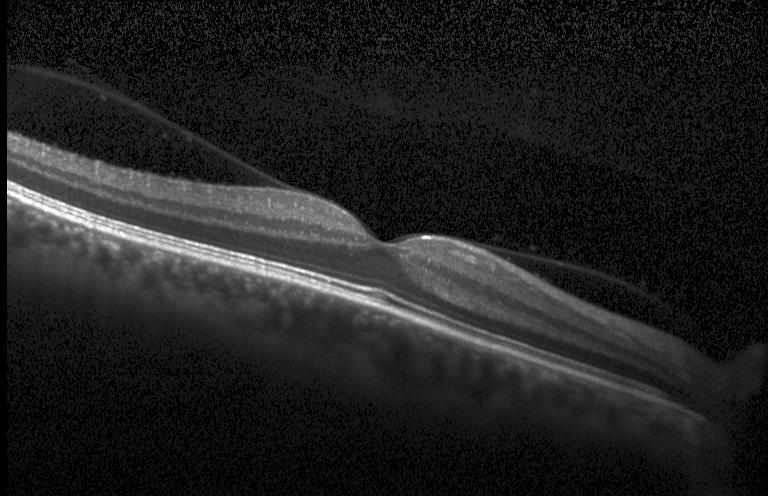

The scan shows no CNV, no DME, and no drusen.